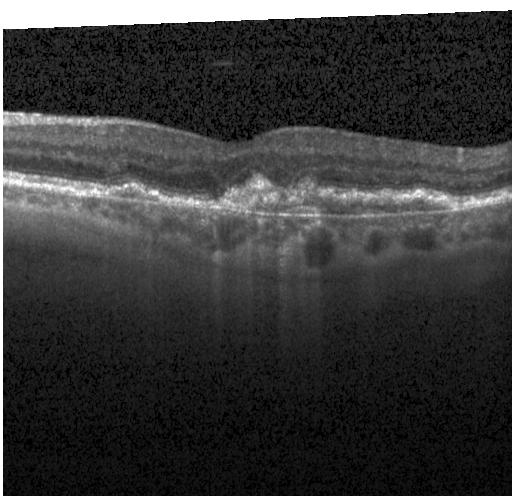
Macular OCT demonstrating CNV.